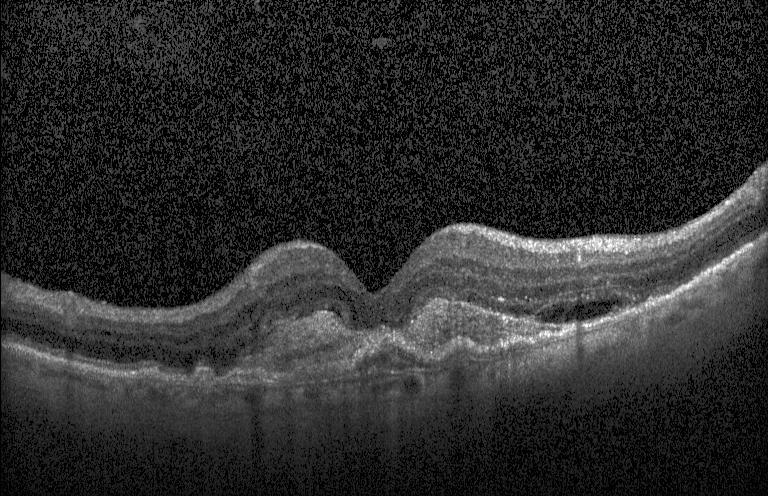
OCT finding: a choroidal neovascular membrane.